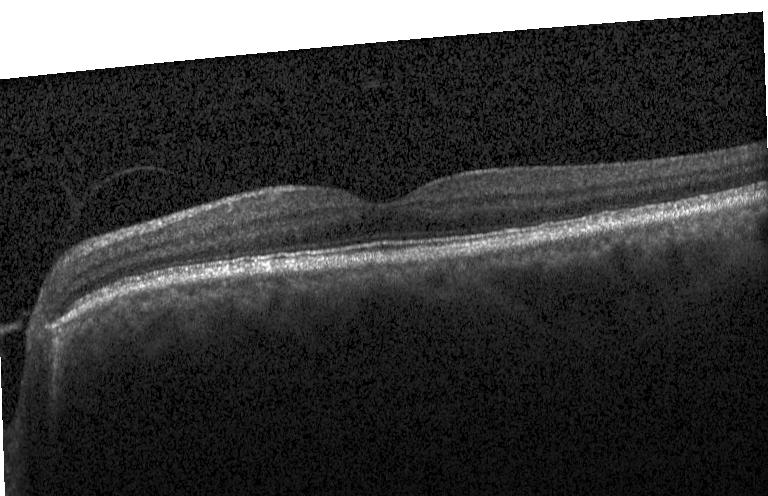 Diagnosis: no CNV, DME, or drusen.